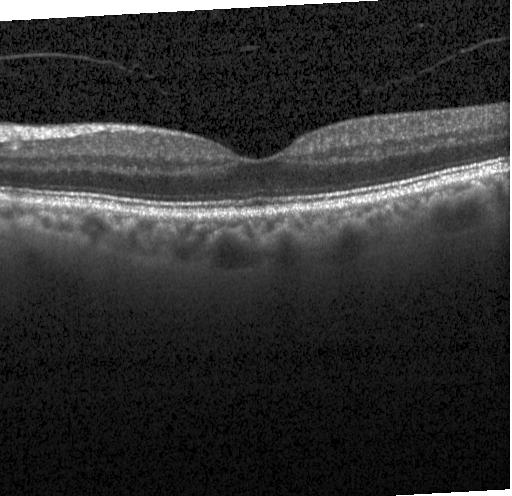 Fovea-centered · optical coherence tomography scan · SD-OCT. Assessment: no CNV, no DME, and no drusen.